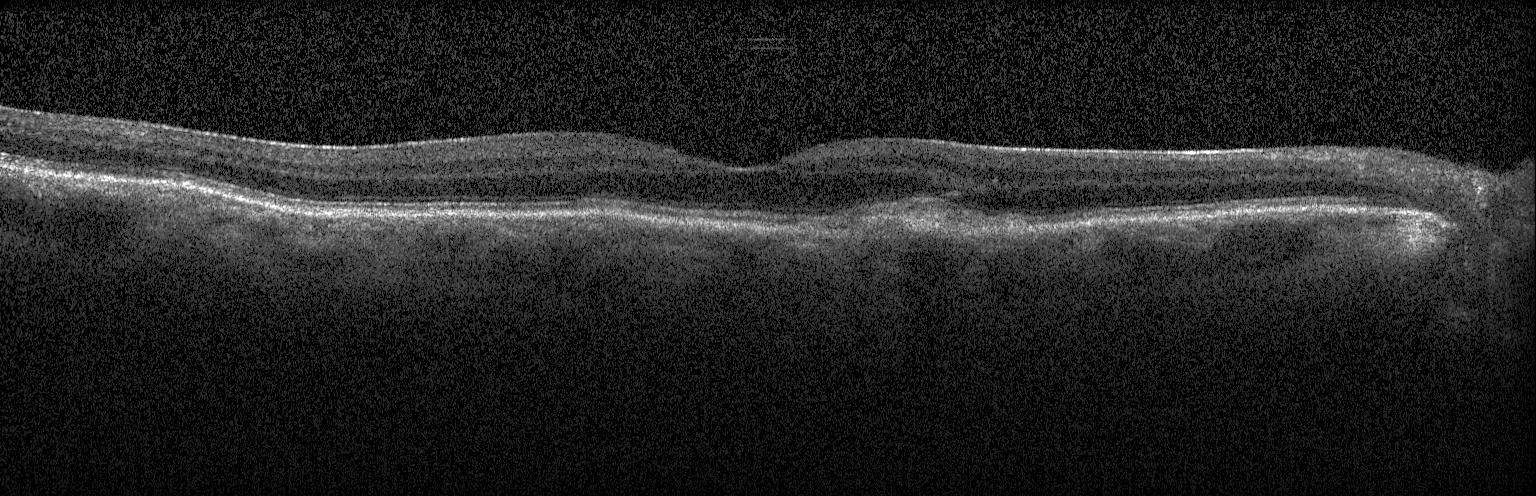 Retinal OCT cross-section showing a choroidal neovascular membrane.